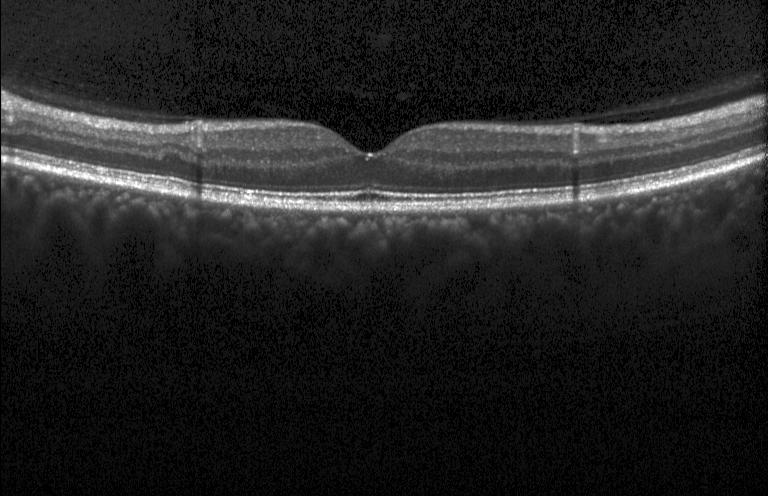

Acquired on a Heidelberg Spectralis. Horizontal scan through the fovea. Spectral-domain OCT. Retinal OCT cross-section
OCT finding: no evidence of choroidal neovascularization, diabetic macular edema, or drusen.